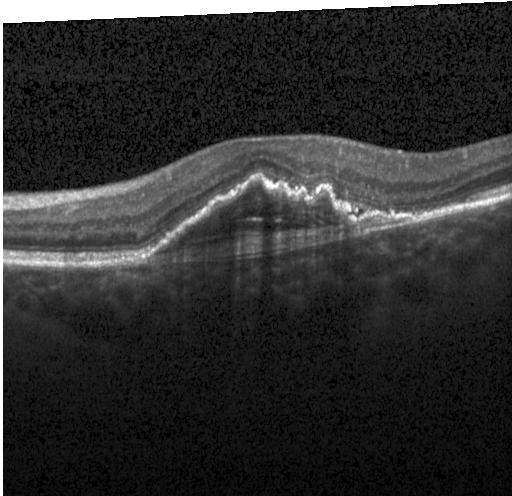
Macular scan; instrument: Heidelberg Spectralis; retinal OCT B-scan. Macular OCT: choroidal neovascularization (CNV).